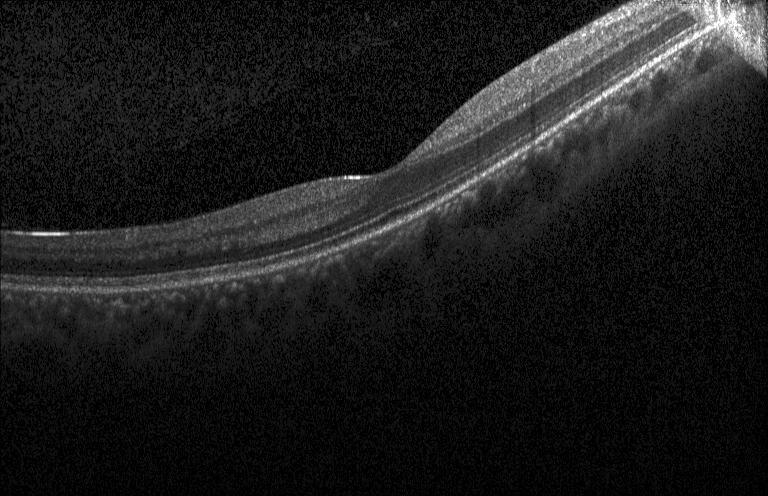 Dx: neither CNV, DME, nor drusen.